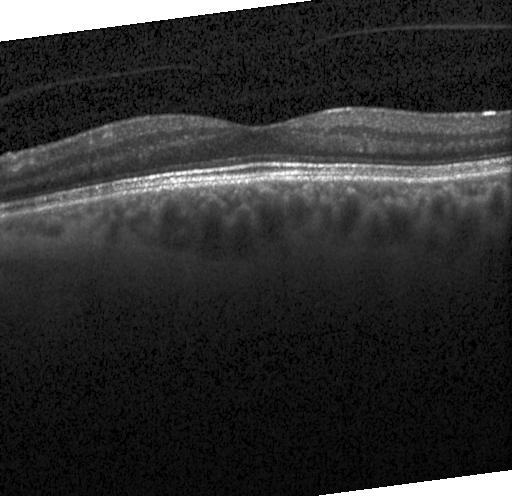
Through the macula; OCT line scan; spectral-domain optical coherence tomography.
The scan shows neither CNV, DME, nor drusen.